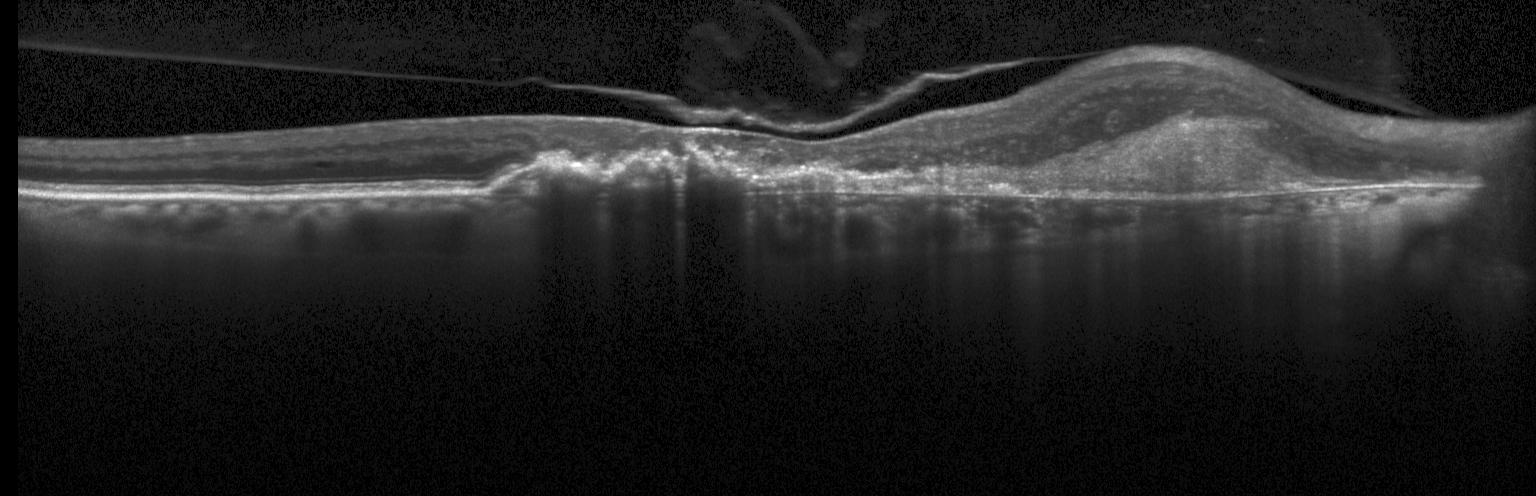

Macular OCT: a choroidal neovascular membrane.